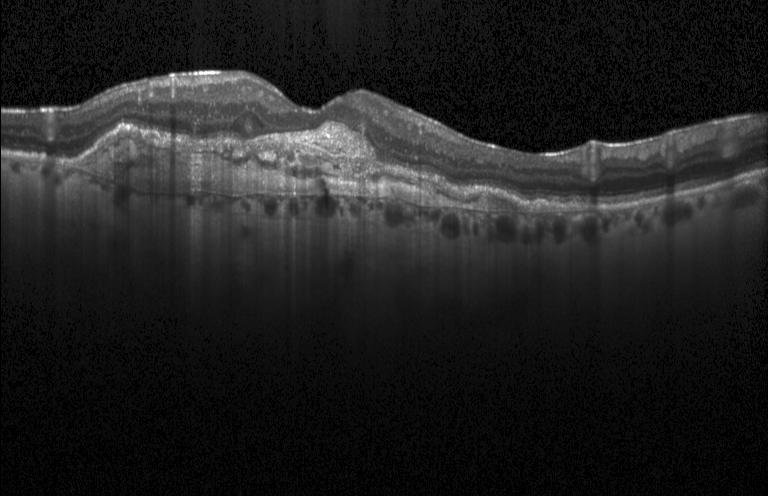 Retinal OCT B-scan, centered on the fovea.
Assessment: choroidal neovascularization (CNV).